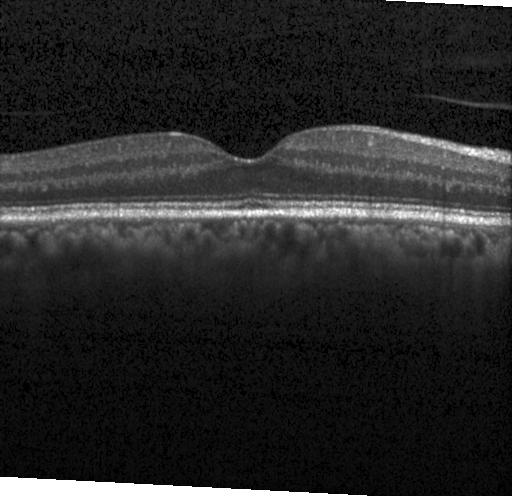
Retinal OCT cross-section. Finding: no choroidal neovascularization, diabetic macular edema, or drusen.